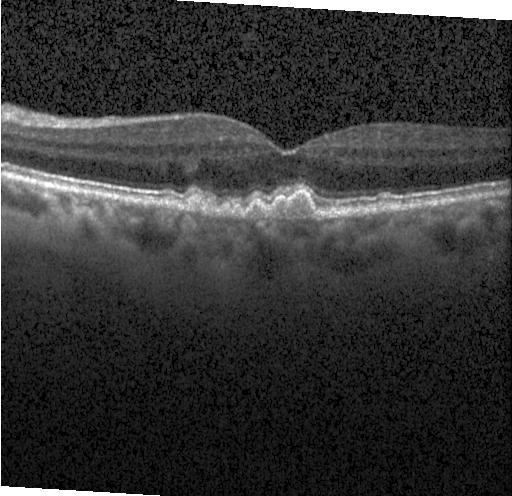
SD-OCT · OCT B-scan · macular scan.
Diagnosis: sub-RPE drusenoid deposits.